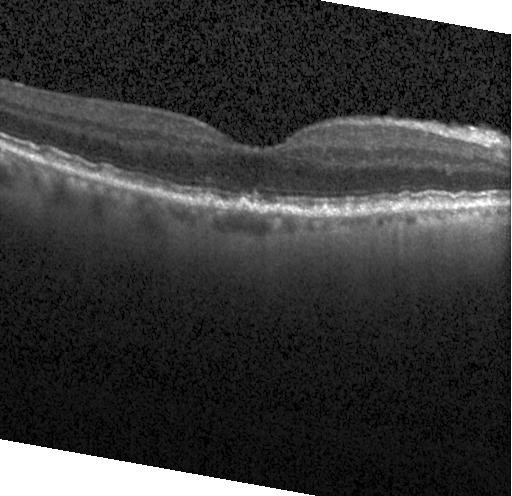
Heidelberg Spectralis; OCT B-scan; centered on the fovea
Dx: drusen.